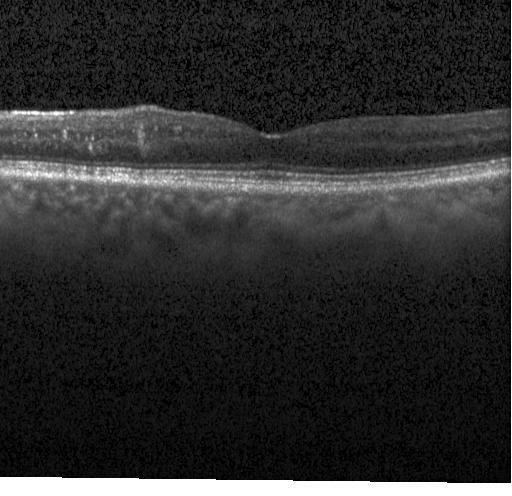

Acquired on a Heidelberg Spectralis. Optical coherence tomography B-scan. Fovea-centered — Diagnosis: no choroidal neovascularization, no diabetic macular edema, and no drusen.